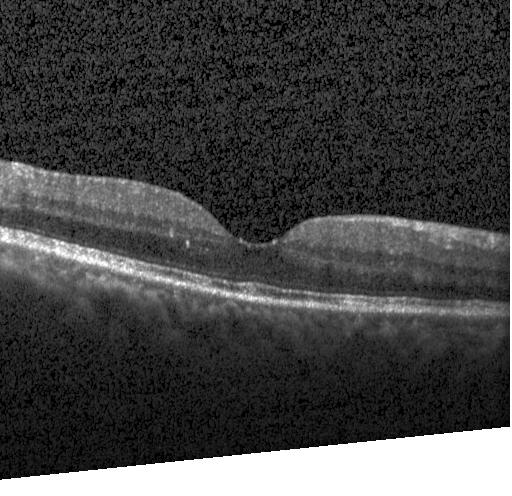 Neither CNV, DME, nor drusen.